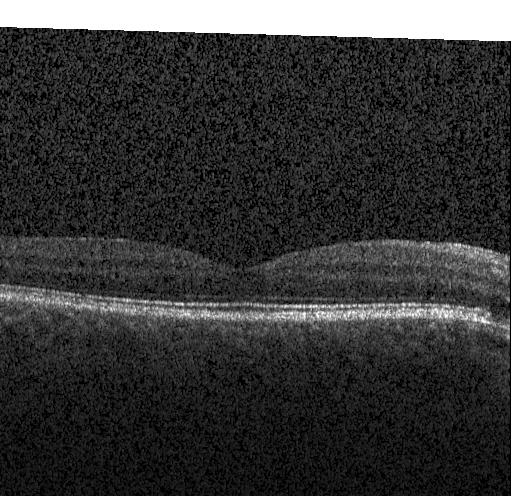

Optical coherence tomography B-scan
The scan shows no choroidal neovascularization, diabetic macular edema, or drusen.